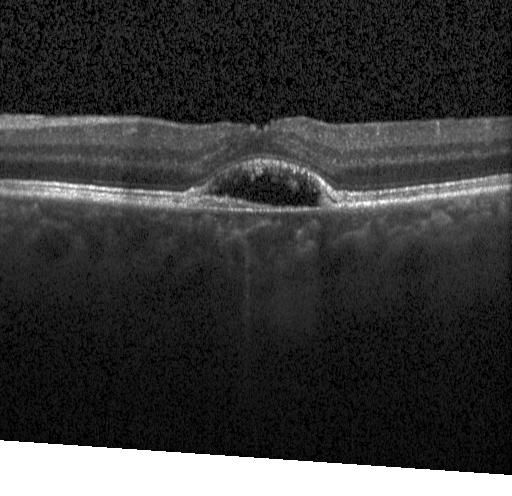

OCT B-scan showing a choroidal neovascular membrane.